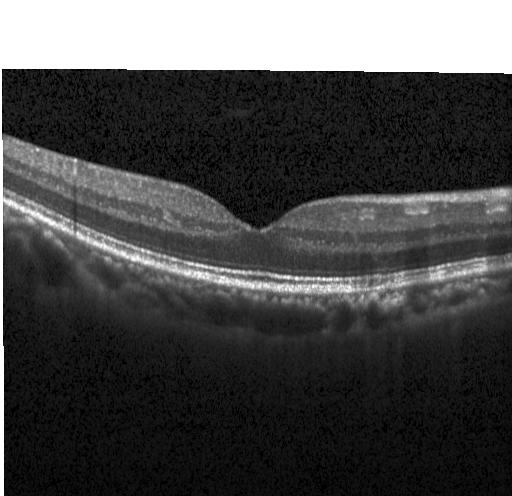
Assessment: no CNV, DME, or drusen.